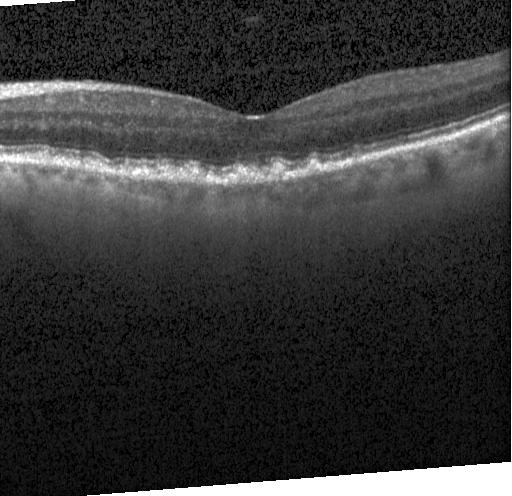 Diagnosis: multiple drusen.